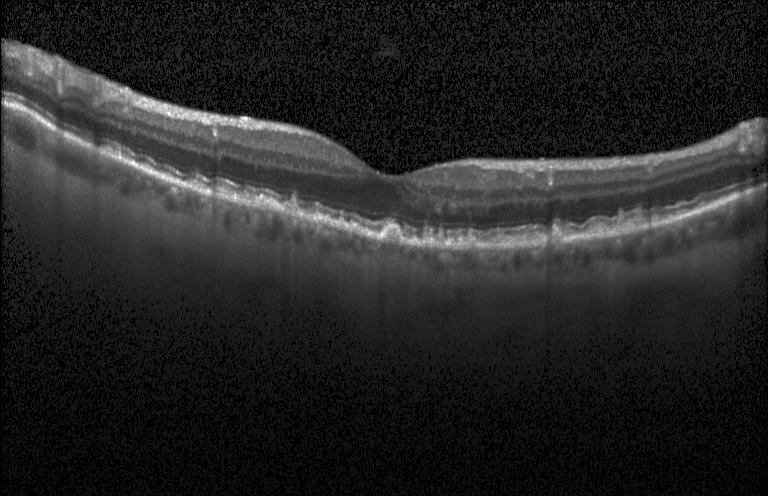

Optical coherence tomography scan; instrument: Heidelberg Spectralis.
Assessment: drusen.